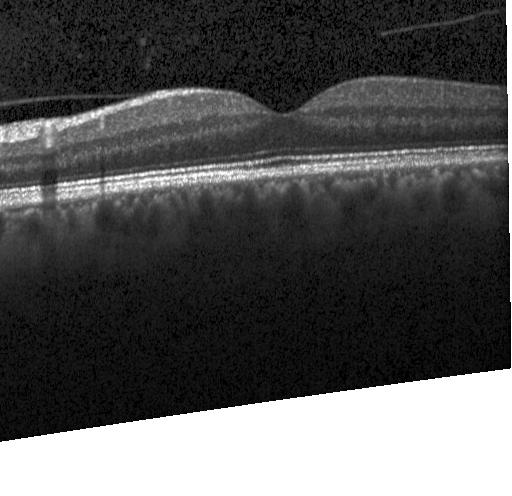 Finding: neither CNV, DME, nor drusen.